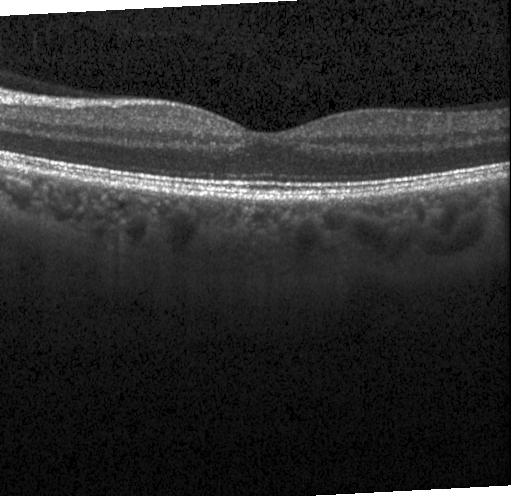
OCT B-scan, through the macula, Heidelberg Spectralis.
Finding: neither choroidal neovascularization, diabetic macular edema, nor drusen.